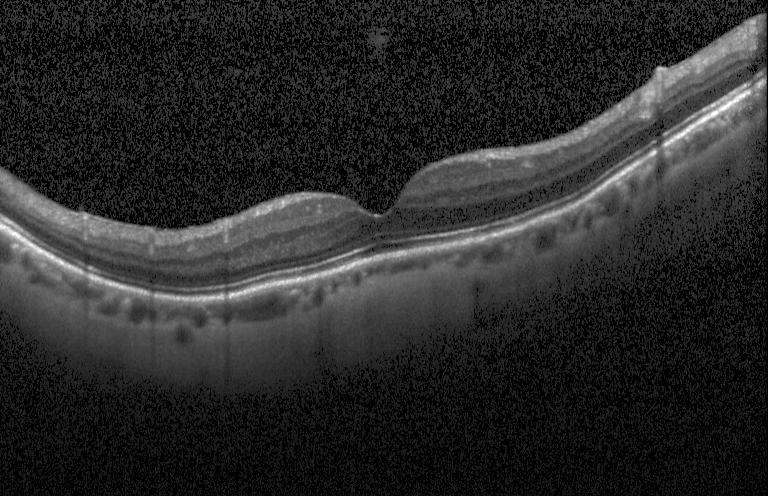

Retinal OCT cross-section · spectral-domain optical coherence tomography.
This B-scan demonstrates neither choroidal neovascularization, diabetic macular edema, nor drusen.